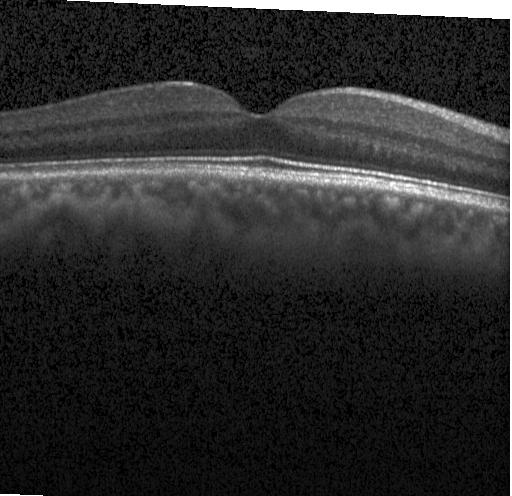
Retinal OCT cross-section. Assessment: no evidence of CNV, DME, or drusen.